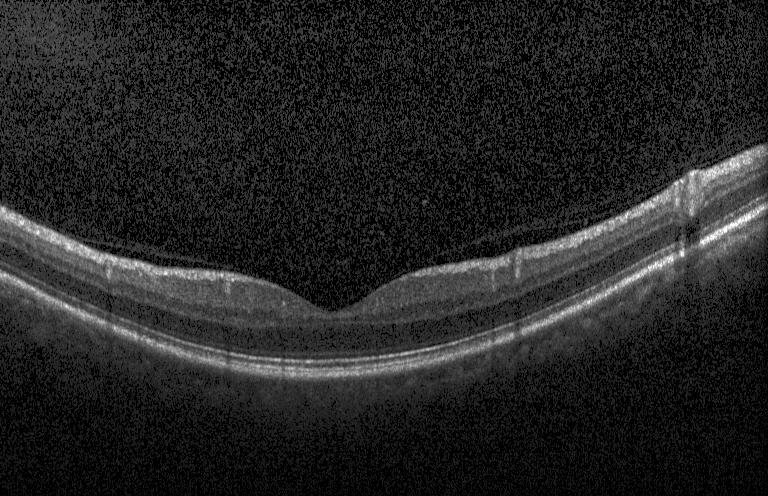 Spectral-domain optical coherence tomography; OCT B-scan — Assessment: no evidence of CNV, DME, or drusen.